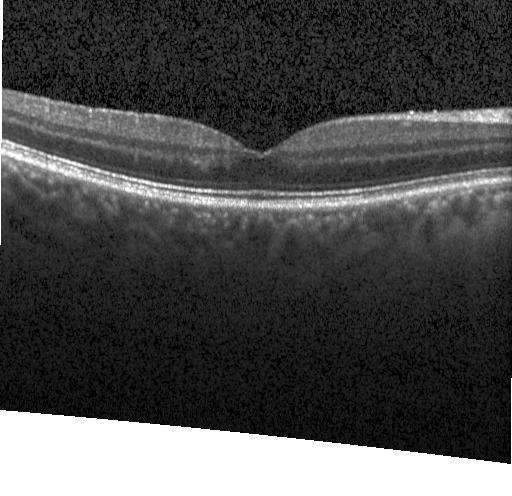

Impression: no choroidal neovascularization, no diabetic macular edema, and no drusen.